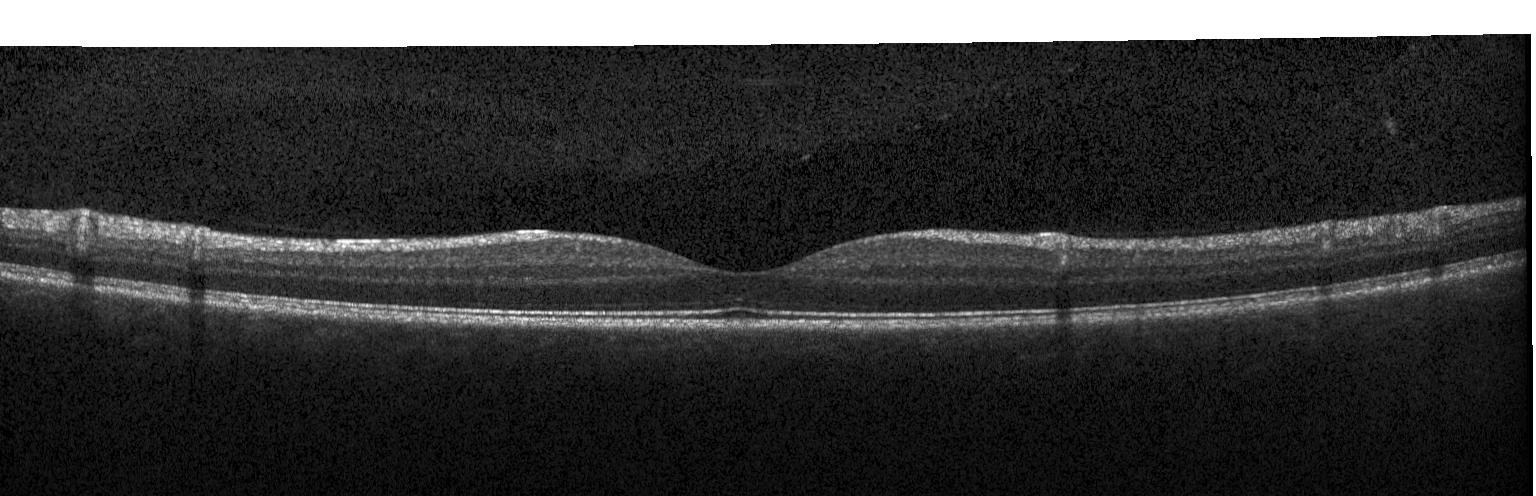
Optical coherence tomography scan. Diagnosis: neither choroidal neovascularization, diabetic macular edema, nor drusen.